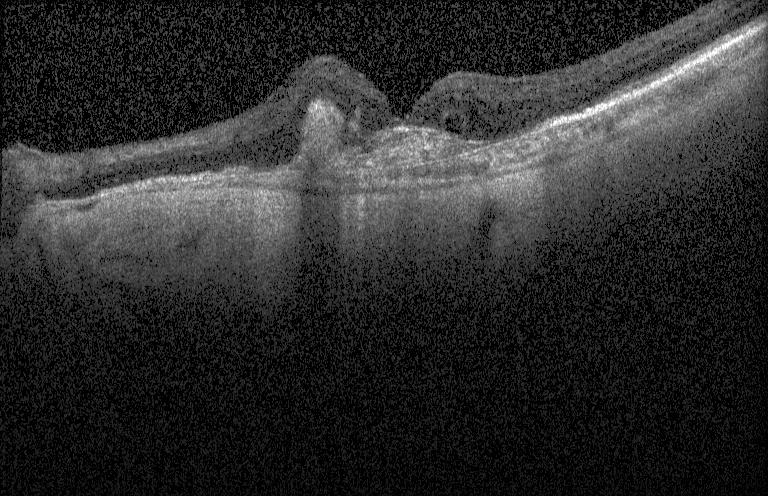
SD-OCT; optical coherence tomography B-scan
The scan shows choroidal neovascularization (CNV).